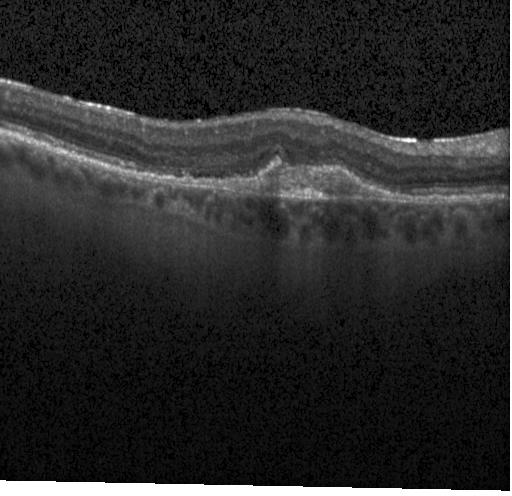 Optical coherence tomography scan. The scan shows choroidal neovascularization (CNV).